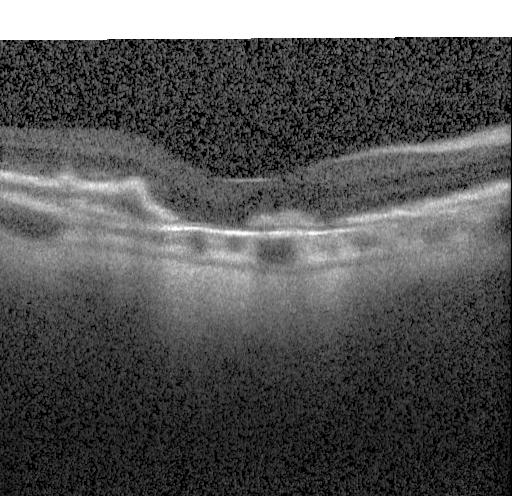

Optical coherence tomography B-scan.
Finding: a choroidal neovascular membrane.